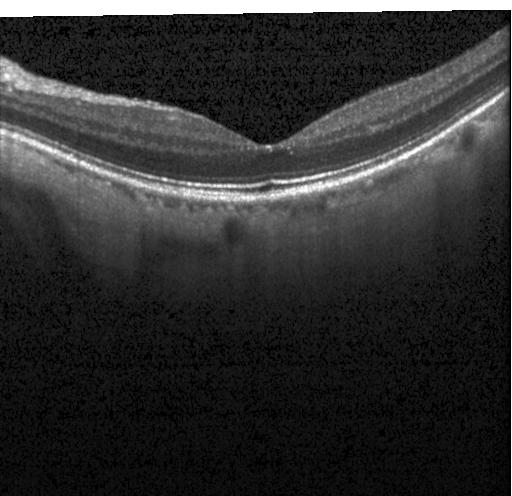

OCT finding: no evidence of choroidal neovascularization, diabetic macular edema, or drusen.